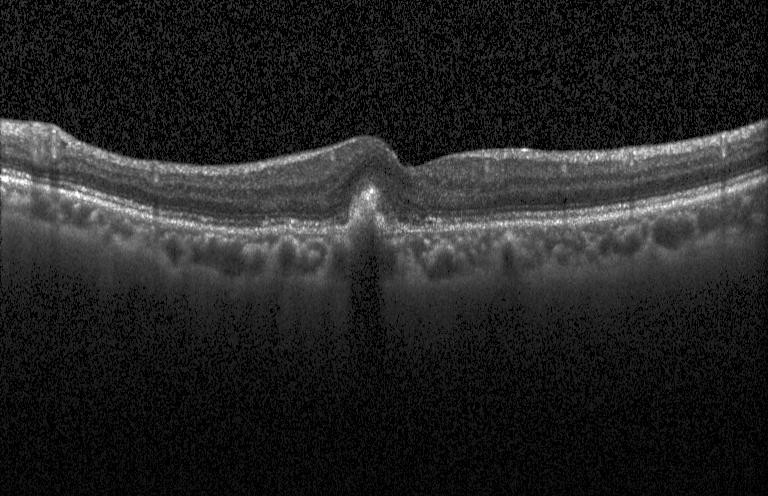
Instrument: Heidelberg Spectralis · OCT B-scan · macular scan · SD-OCT
Diagnosis: a choroidal neovascular membrane.